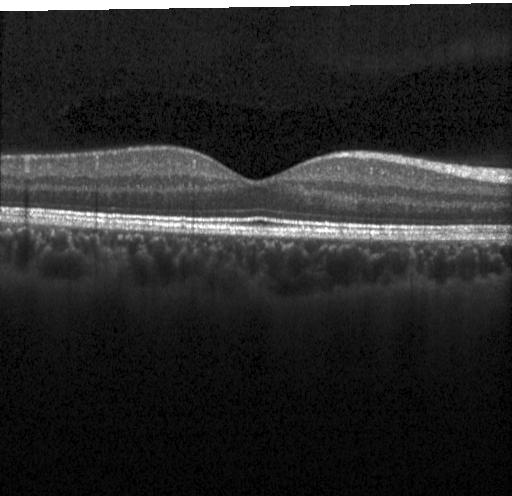
OCT B-scan showing no evidence of choroidal neovascularization, diabetic macular edema, or drusen.